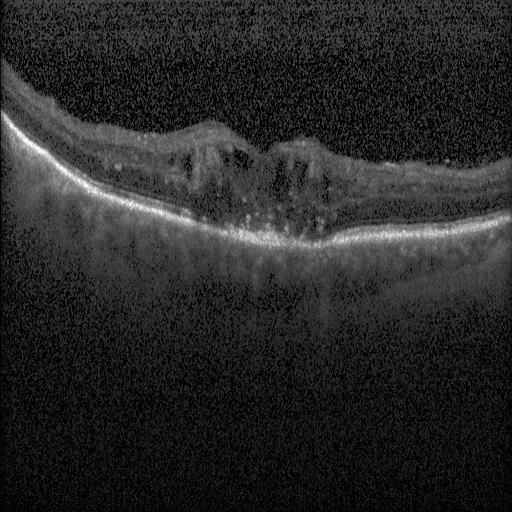 Spectral-domain OCT · instrument: Heidelberg Spectralis · optical coherence tomography B-scan. This B-scan demonstrates DME.